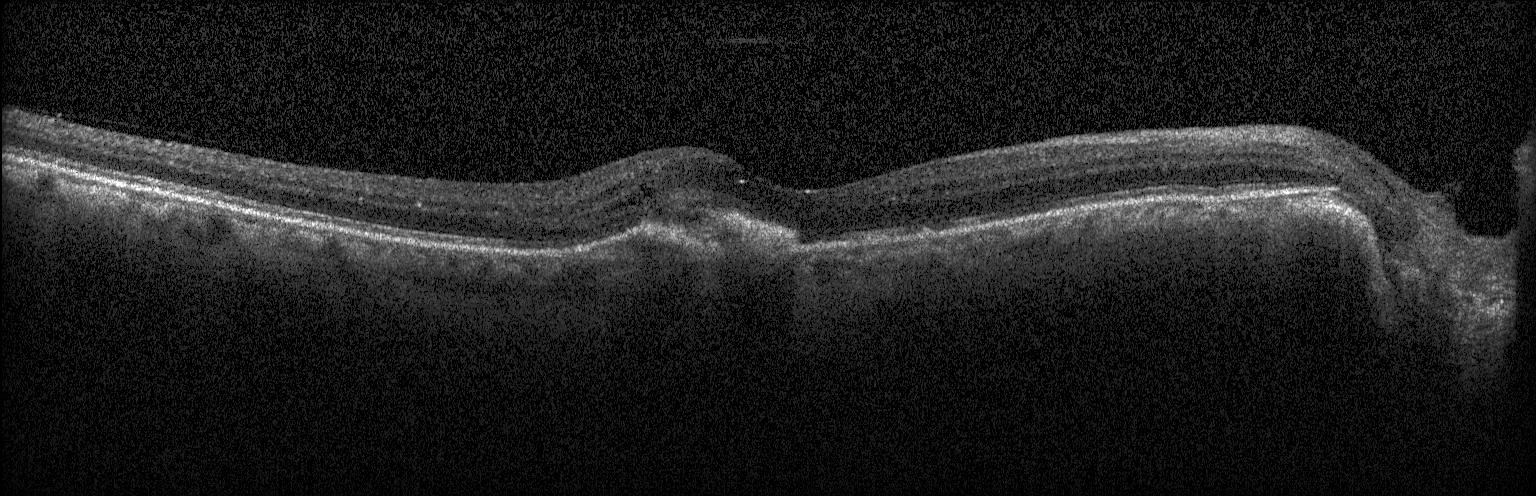
Retinal OCT cross-section — The scan shows a choroidal neovascular membrane.